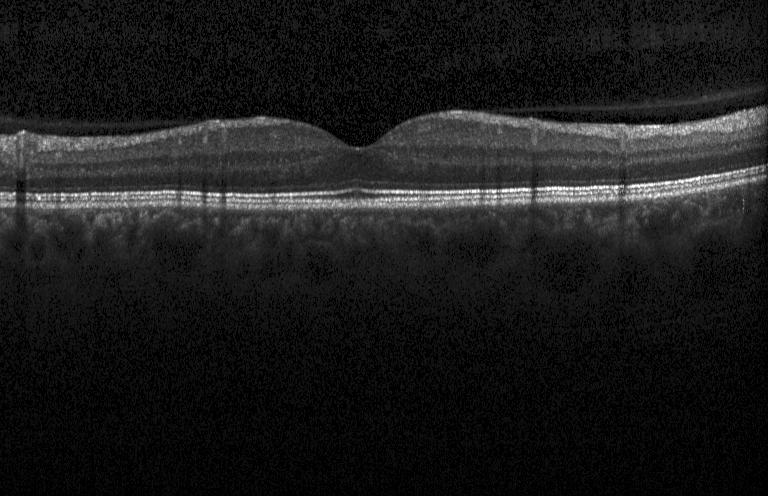

Diagnosis: no CNV, no DME, and no drusen.